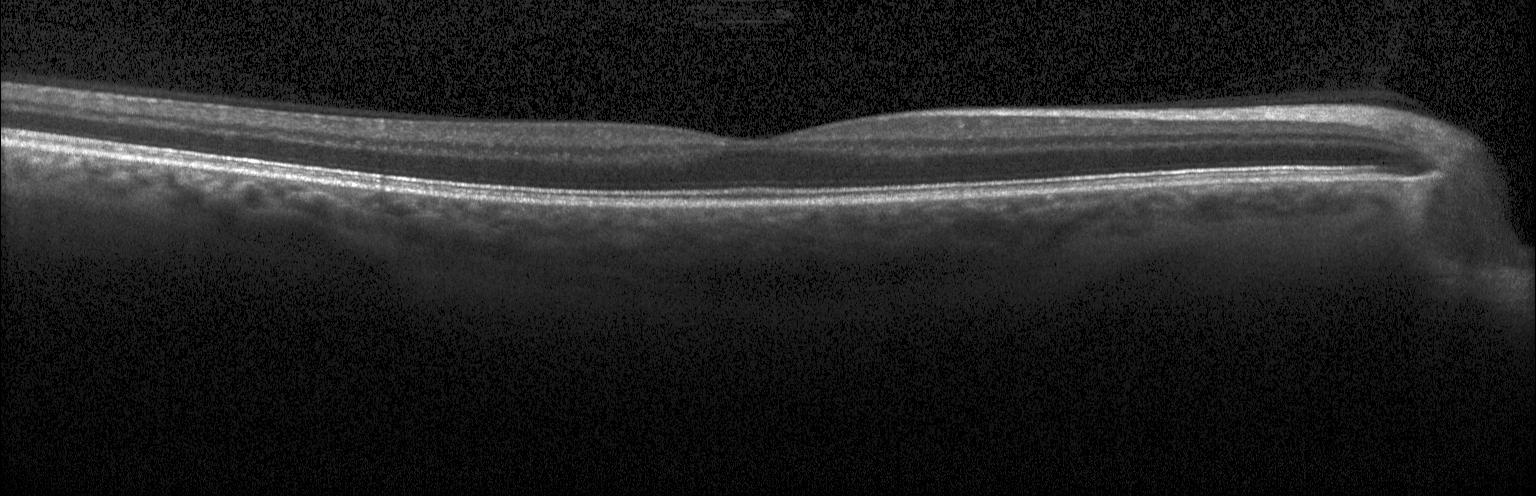

Retinal OCT B-scan · spectral-domain OCT
Diagnosis: no evidence of CNV, DME, or drusen.